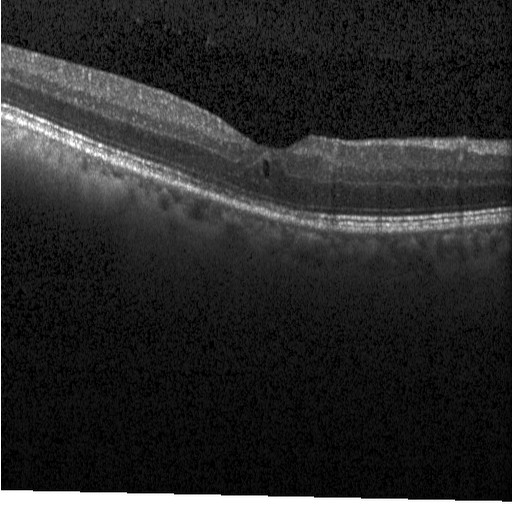
OCT B-scan. Assessment: DME.